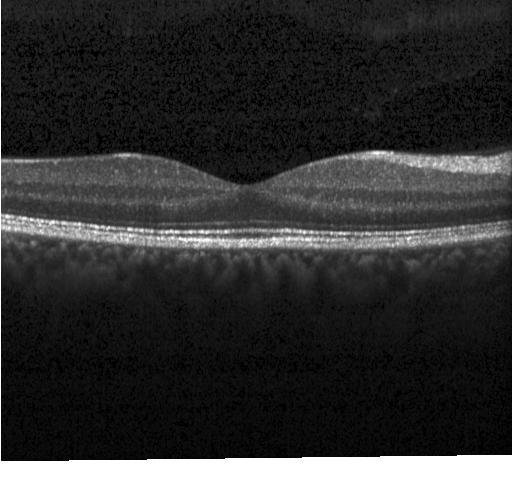
Finding: no choroidal neovascularization, no diabetic macular edema, and no drusen.